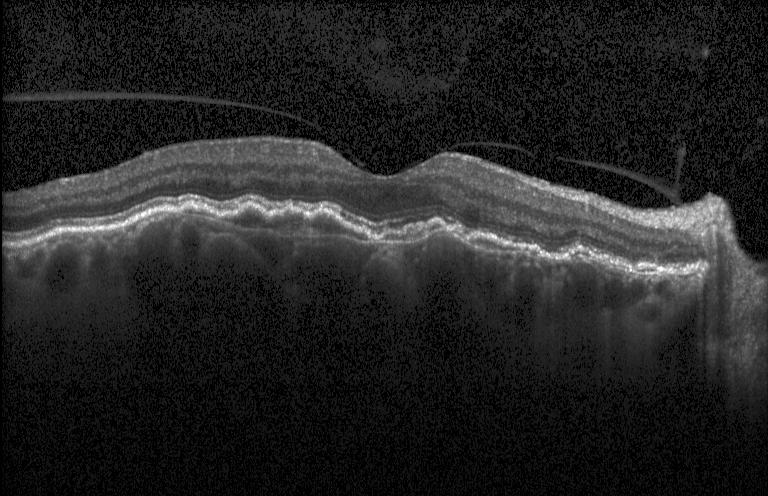

Centered on the fovea. Optical coherence tomography B-scan — Impression: a choroidal neovascular membrane.